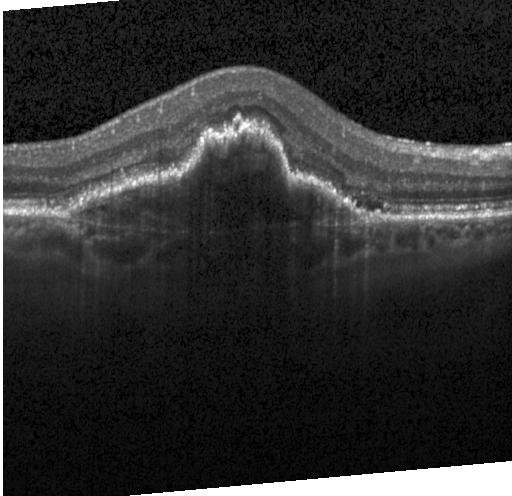

Centered on the fovea · spectral-domain optical coherence tomography · Heidelberg Spectralis · OCT line scan. Macular OCT: a choroidal neovascular membrane.